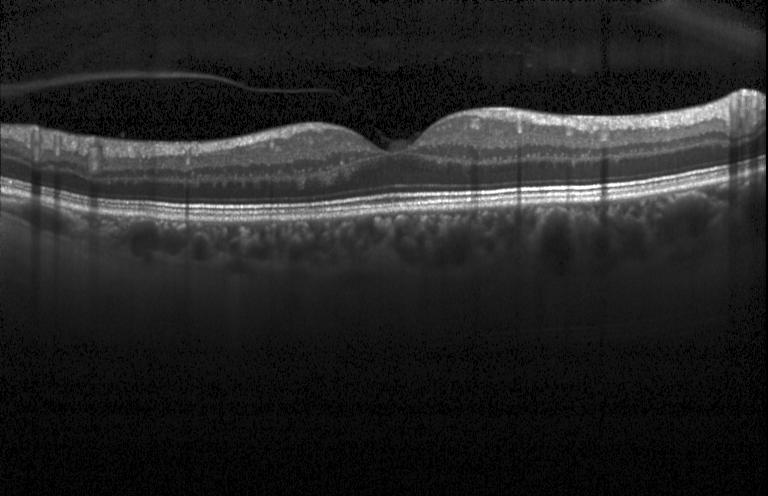 Instrument: Heidelberg Spectralis. Spectral-domain OCT. Macular scan. Optical coherence tomography scan.
Finding: no CNV, DME, or drusen.